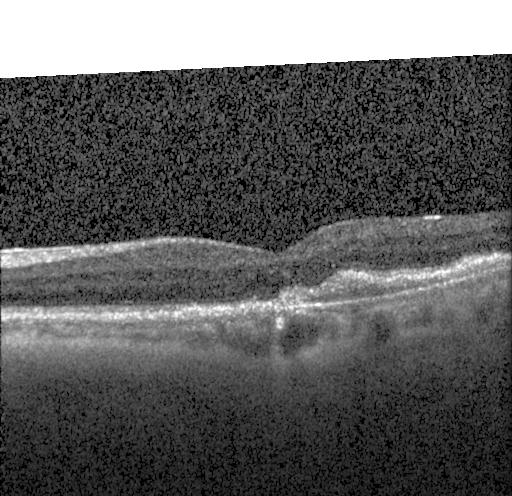

The scan shows a choroidal neovascular membrane.